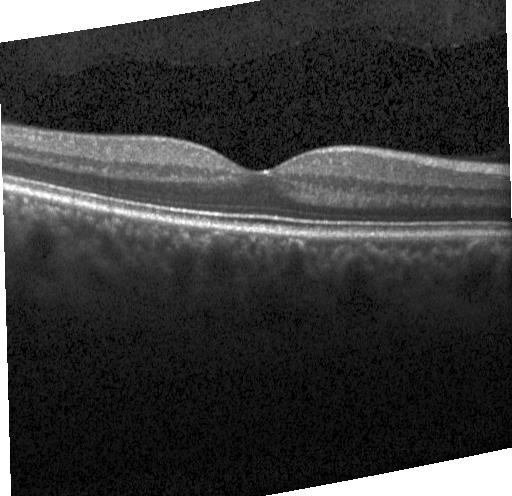 OCT B-scan · spectral-domain OCT · through the macula · Heidelberg Spectralis OCT system — Diagnosis: no evidence of CNV, DME, or drusen.